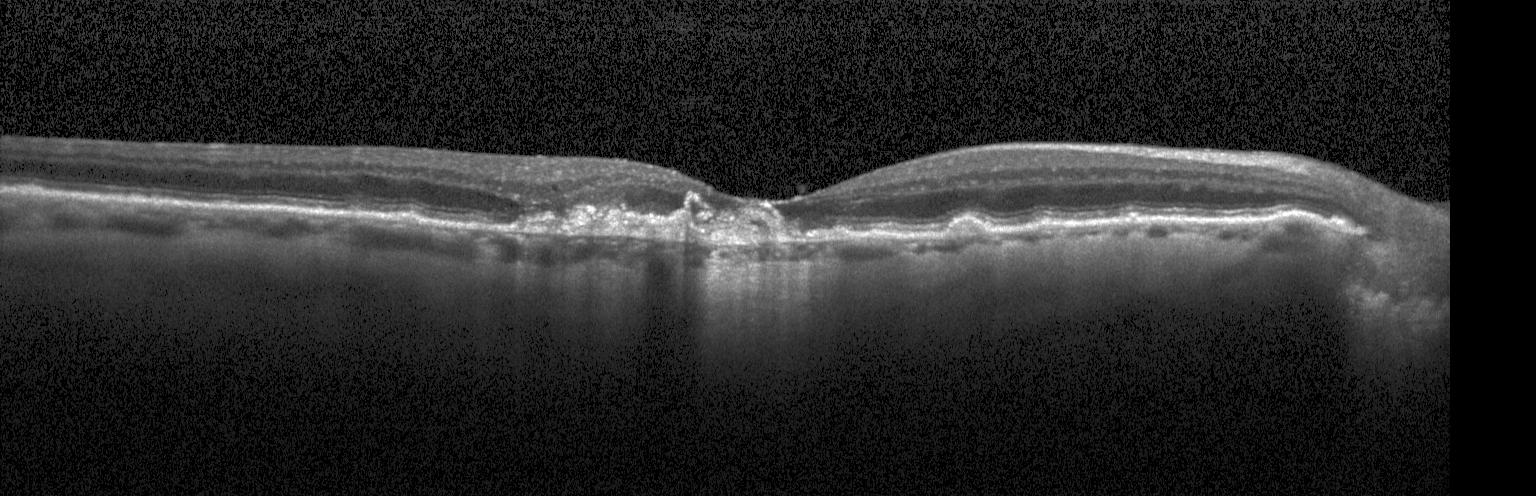
Retinal OCT B-scan. The scan shows a choroidal neovascular membrane.